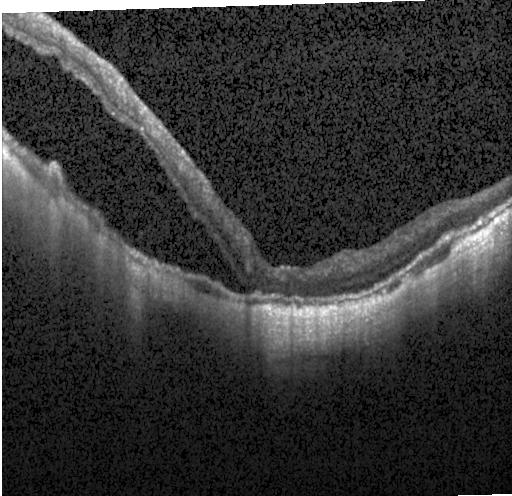

Acquired on a Heidelberg Spectralis; optical coherence tomography scan; SD-OCT — Impression: choroidal neovascularization.